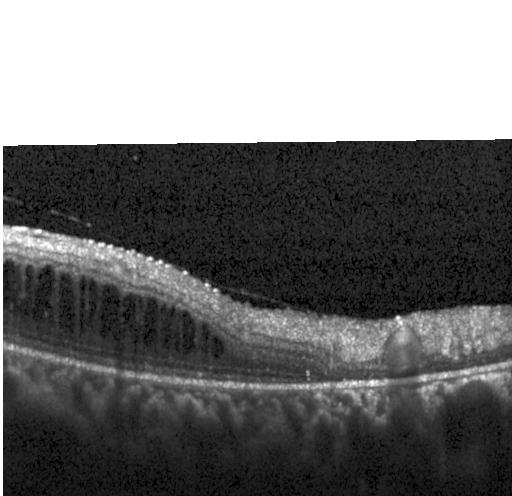
Optical coherence tomography B-scan. Diagnosis: DME.